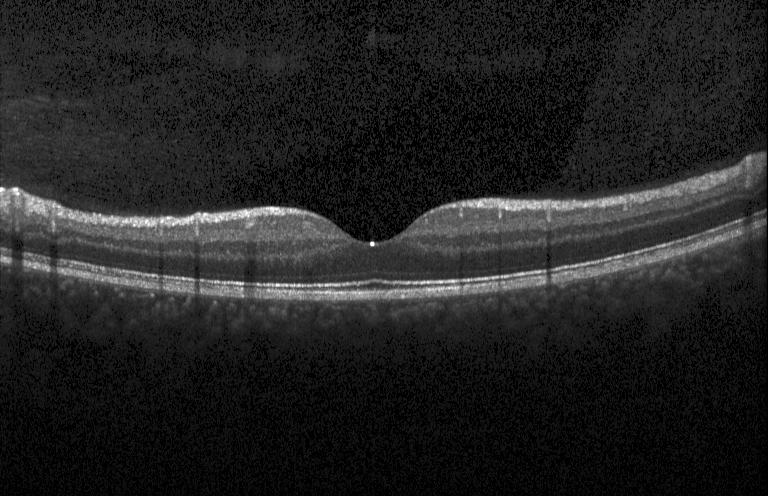

Spectral-domain OCT B-scan: neither CNV, DME, nor drusen.